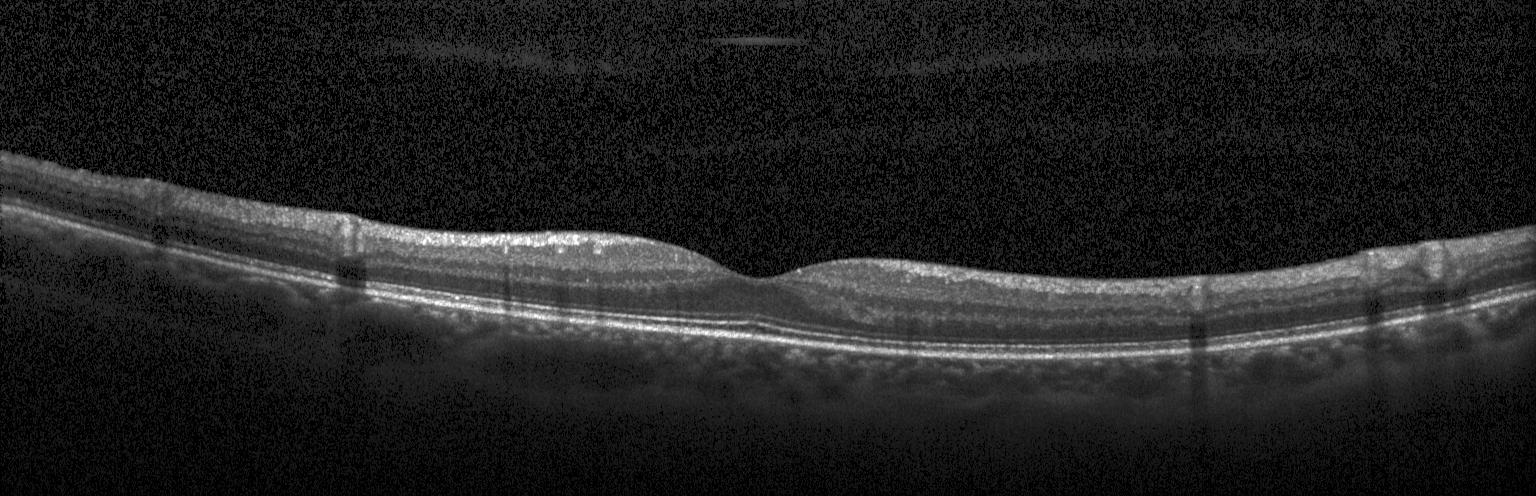

Assessment: no evidence of choroidal neovascularization, diabetic macular edema, or drusen.